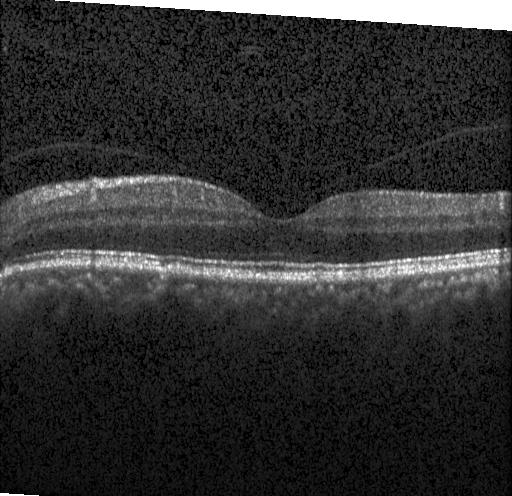

SD-OCT. Optical coherence tomography scan. Fovea-centered — OCT finding: no choroidal neovascularization, no diabetic macular edema, and no drusen.